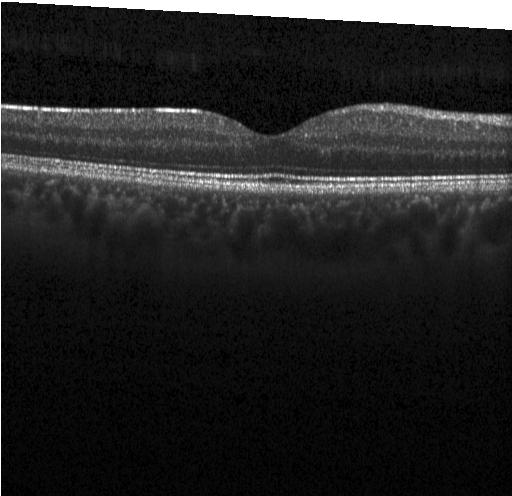 Finding: neither CNV, DME, nor drusen.